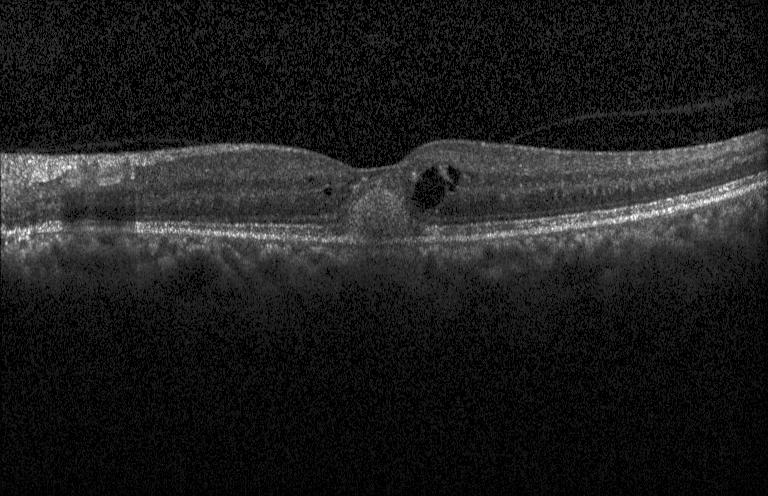

Retinal OCT B-scan.
The scan shows CNV.